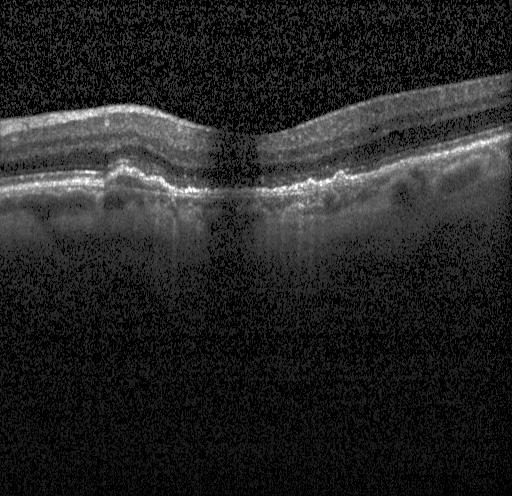
Dx: a choroidal neovascular membrane.